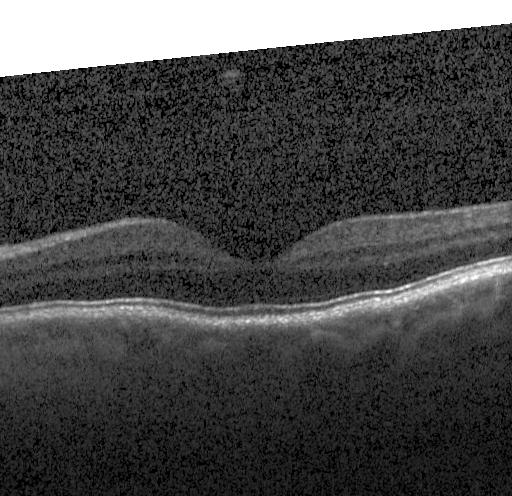 Retinal OCT B-scan
This B-scan demonstrates no choroidal neovascularization, no diabetic macular edema, and no drusen.